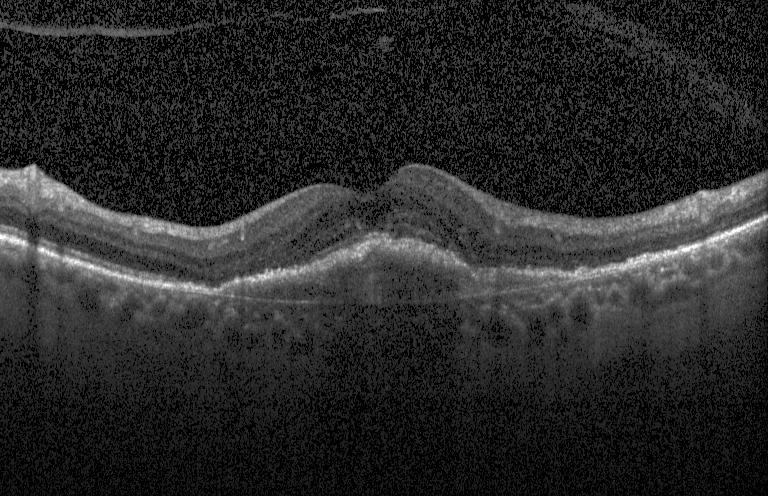

Spectral-domain optical coherence tomography · fovea-centered · acquired on a Heidelberg Spectralis · OCT B-scan. Finding: CNV.